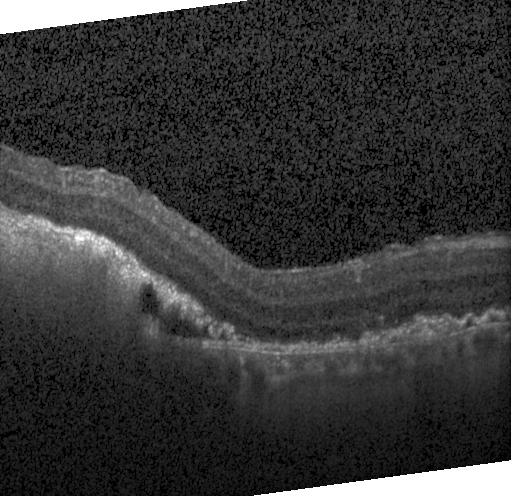 Optical coherence tomography B-scan. The scan shows CNV.